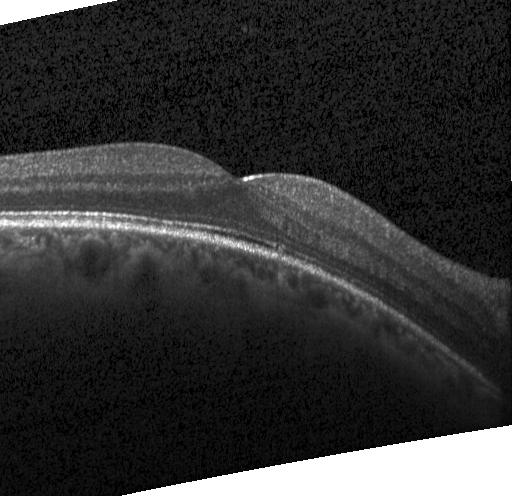
This B-scan demonstrates no CNV, no DME, and no drusen.